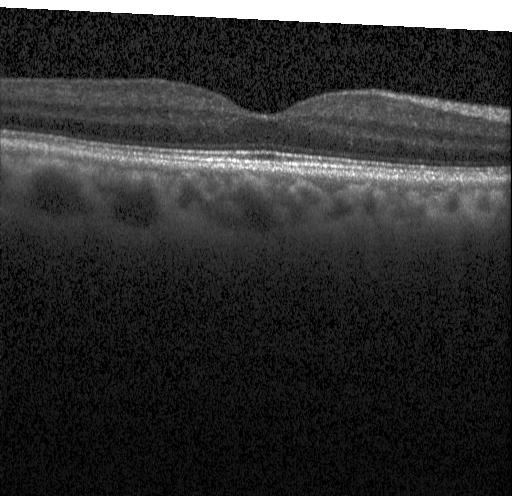

Heidelberg Spectralis OCT system · optical coherence tomography B-scan. OCT finding: neither choroidal neovascularization, diabetic macular edema, nor drusen.